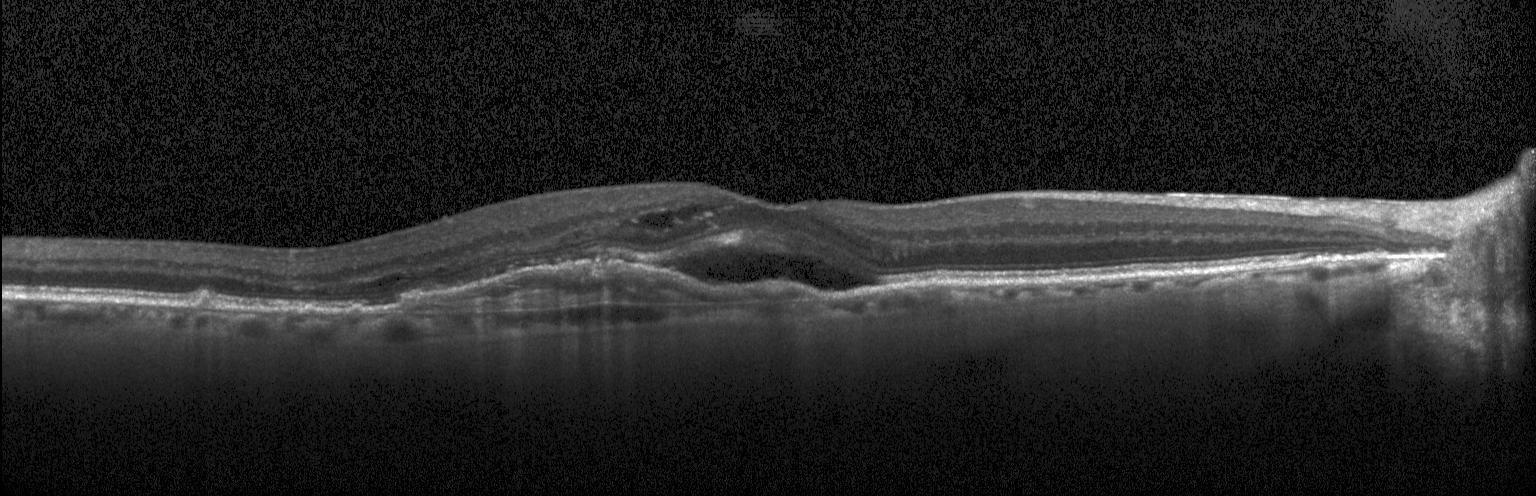 Dx: choroidal neovascularization (CNV).